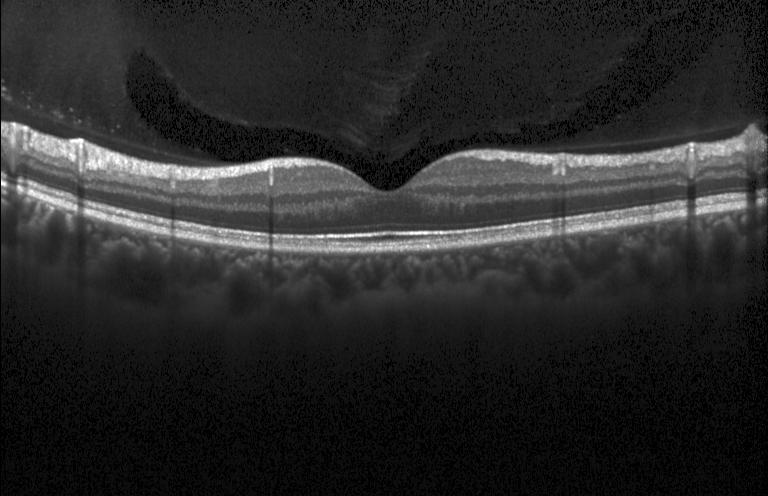
Macular scan, retinal OCT B-scan — Impression: no CNV, DME, or drusen.